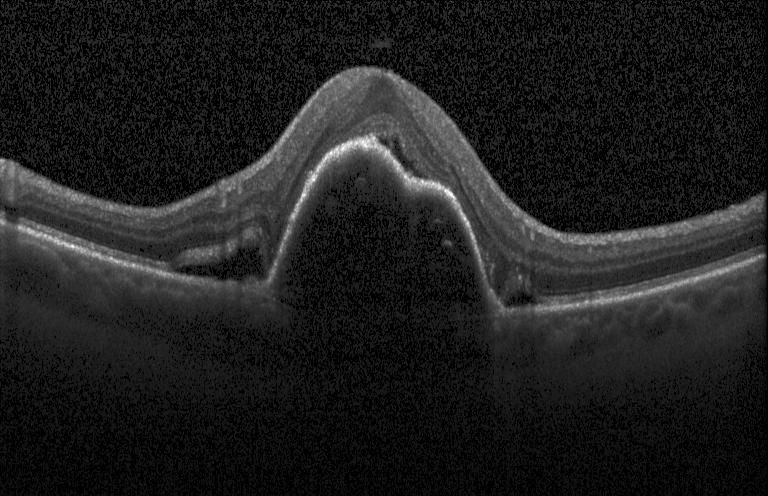 Retinal OCT B-scan; through the macula; spectral-domain OCT; acquired on a Heidelberg Spectralis
Dx: choroidal neovascularization.